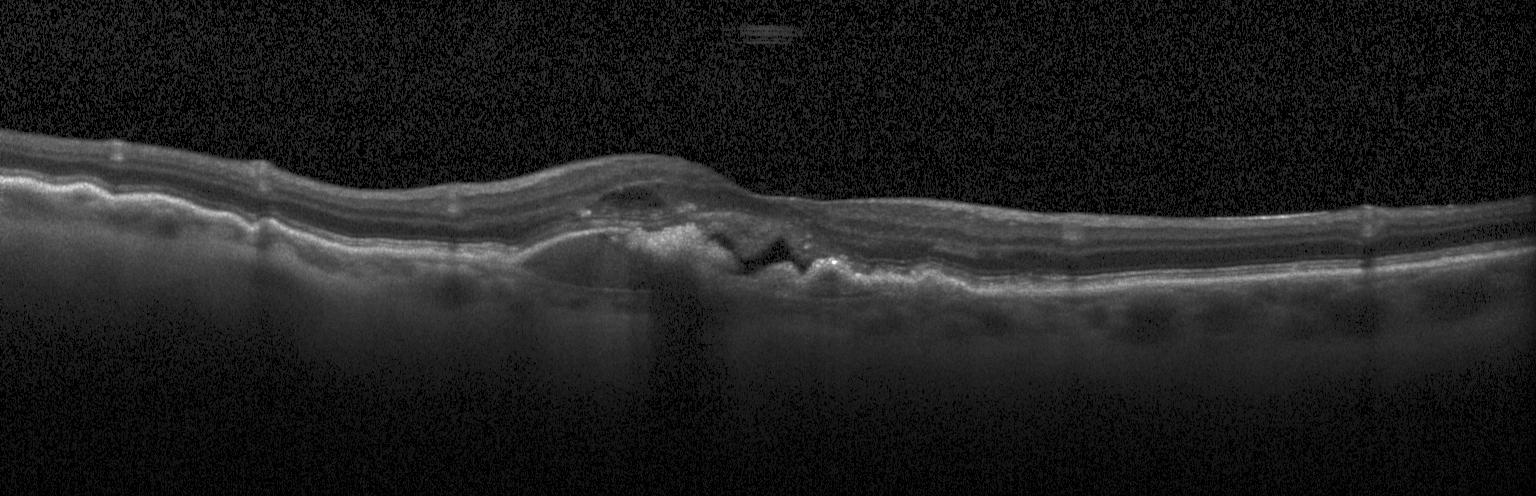

Finding: choroidal neovascularization (CNV).